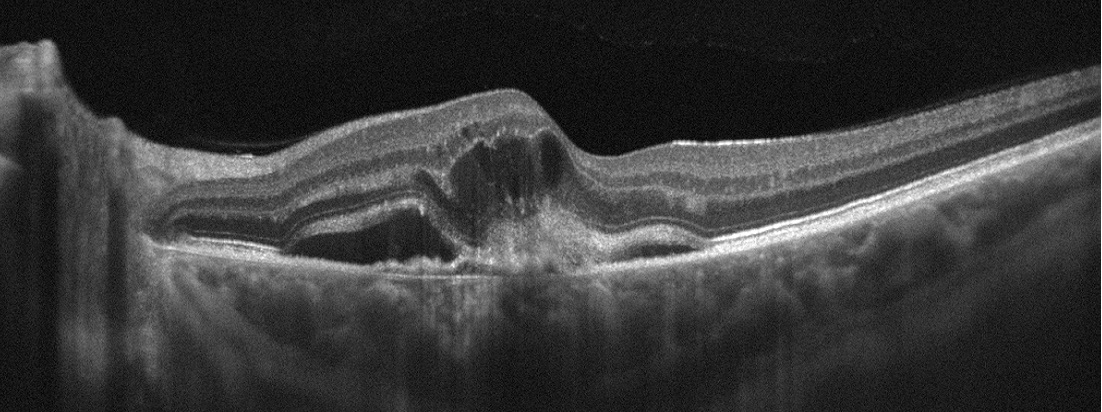

The scan shows age-related macular degeneration.